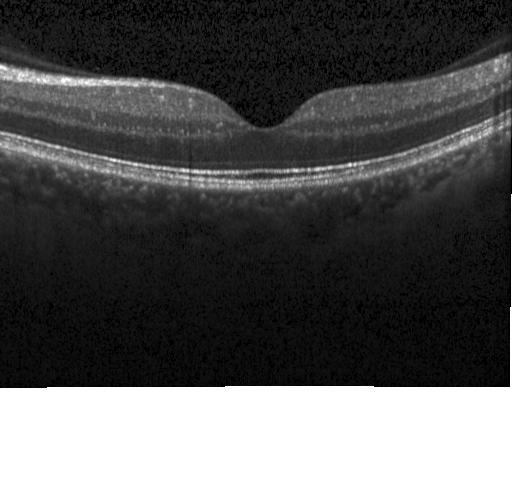 Retinal OCT cross-section showing neither CNV, DME, nor drusen.